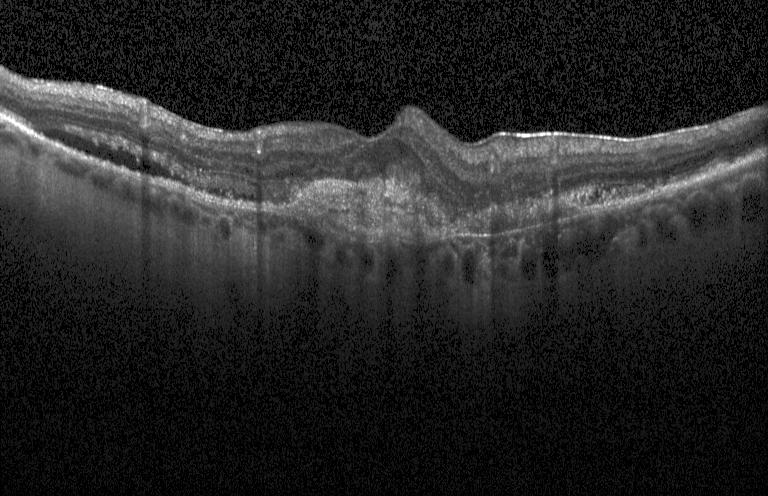 Assessment: choroidal neovascularization (CNV).